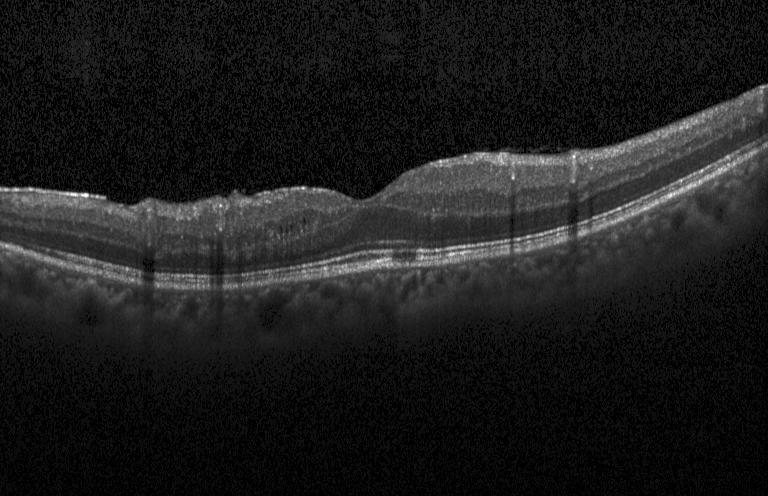 Retinal OCT cross-section.
Diabetic macular edema.